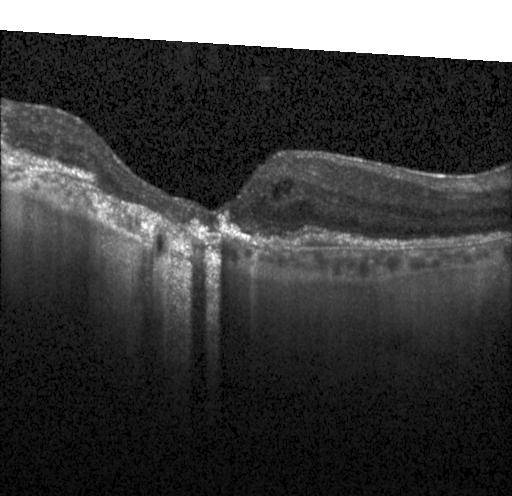
Through the macula; acquired on a Heidelberg Spectralis; optical coherence tomography scan — A choroidal neovascular membrane.